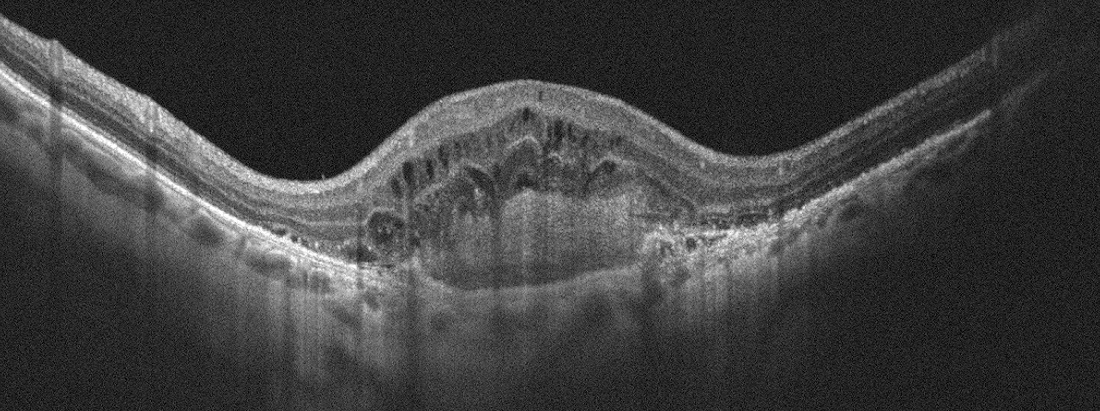 Macular OCT: age-related macular degeneration.